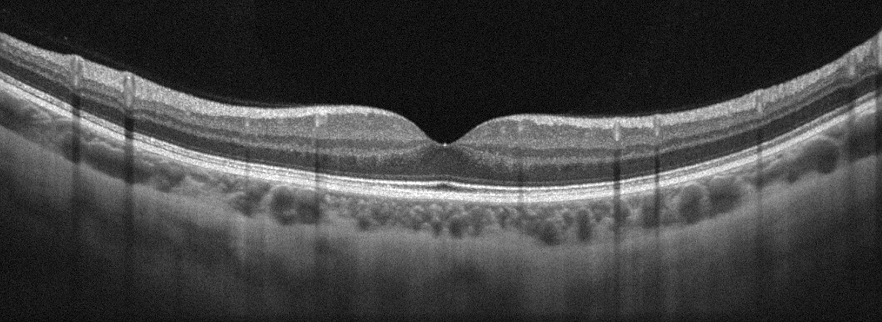

Oculus dexter. Macular scan. Retinal OCT B-scan. Acquired on an Optovue Avanti RTVue XR.
This B-scan demonstrates no evidence of AMD, DME, ERM, RAO, RVO, or VID.